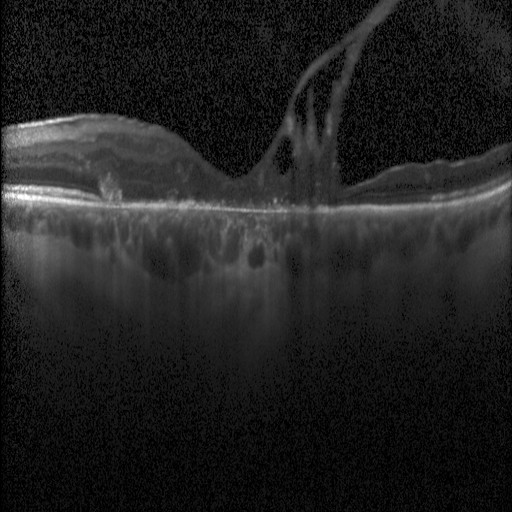

Fovea-centered · spectral-domain OCT · optical coherence tomography B-scan.
Impression: diabetic macular edema (DME).